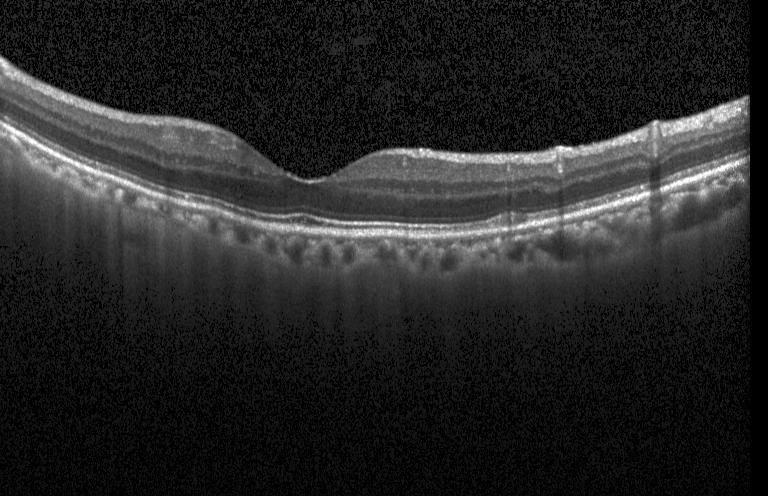

This B-scan demonstrates no choroidal neovascularization, diabetic macular edema, or drusen.